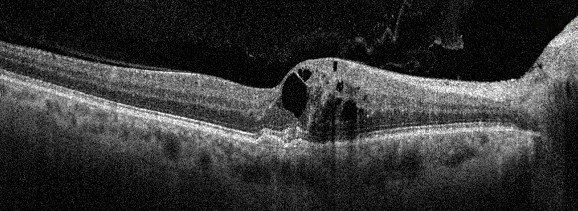 OCT B-scan
The scan shows RVO.